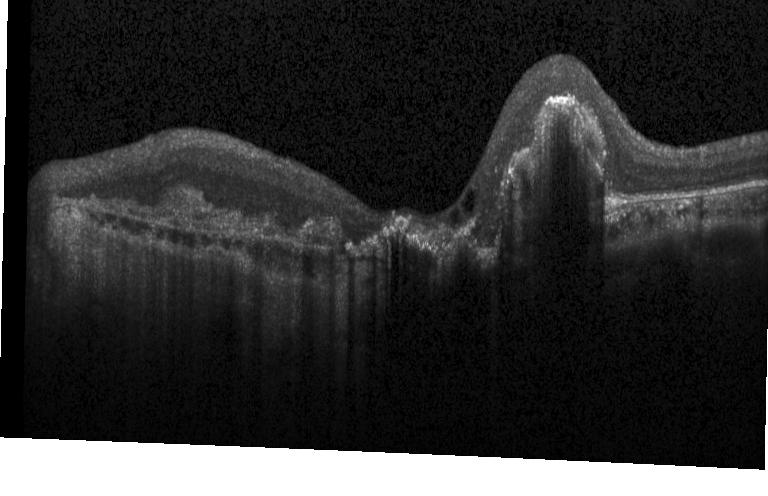 OCT line scan. Spectral-domain OCT — Finding: a choroidal neovascular membrane.